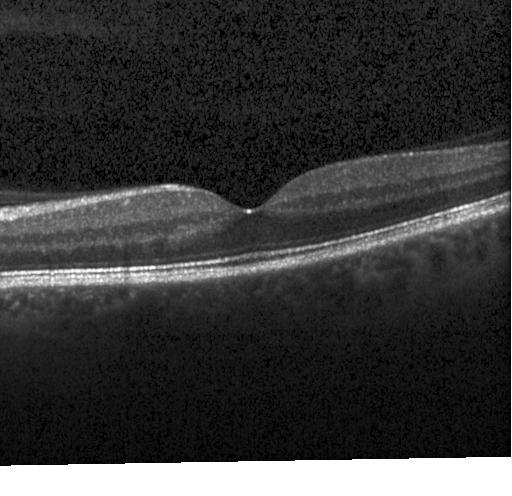
Spectral-domain optical coherence tomography · Heidelberg Spectralis · fovea-centered · OCT line scan.
The scan shows neither choroidal neovascularization, diabetic macular edema, nor drusen.